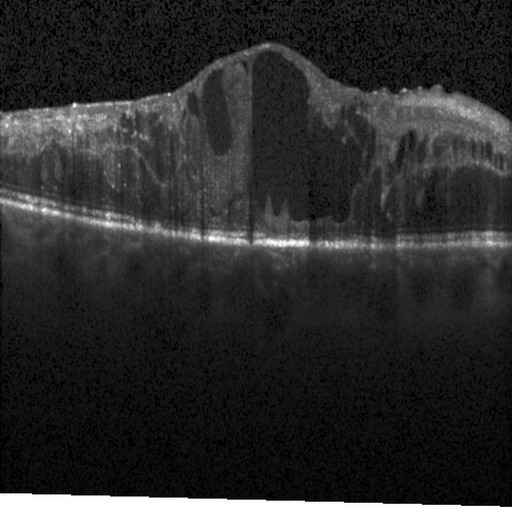 Centered on the fovea, instrument: Heidelberg Spectralis, retinal OCT B-scan, spectral-domain OCT.
This B-scan demonstrates diabetic macular edema.